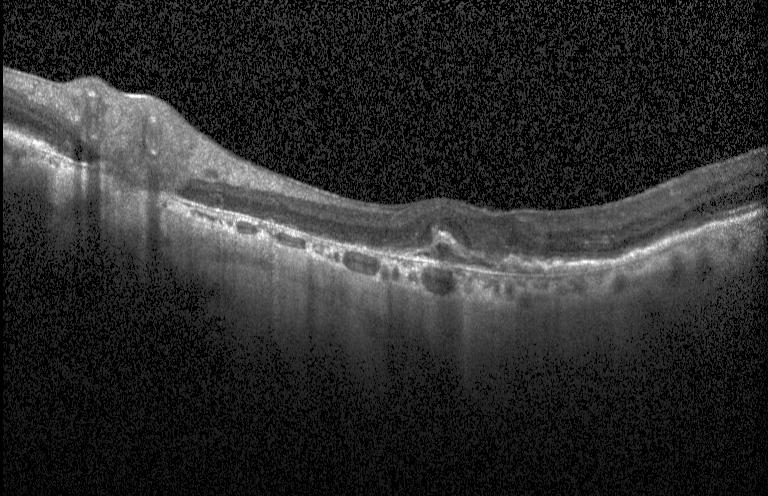 Diagnosis: choroidal neovascularization.